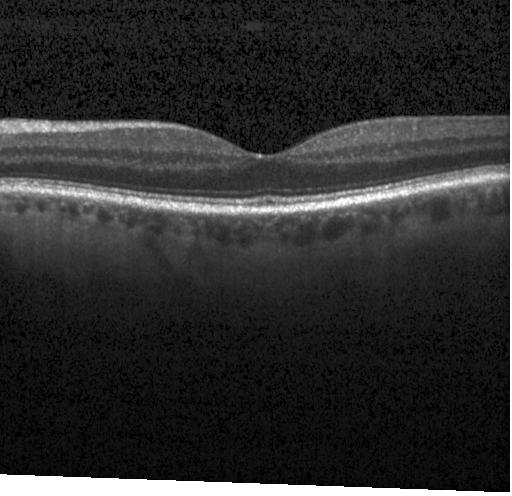

Retinal OCT B-scan · Heidelberg Spectralis · spectral-domain OCT.
Impression: no choroidal neovascularization, diabetic macular edema, or drusen.